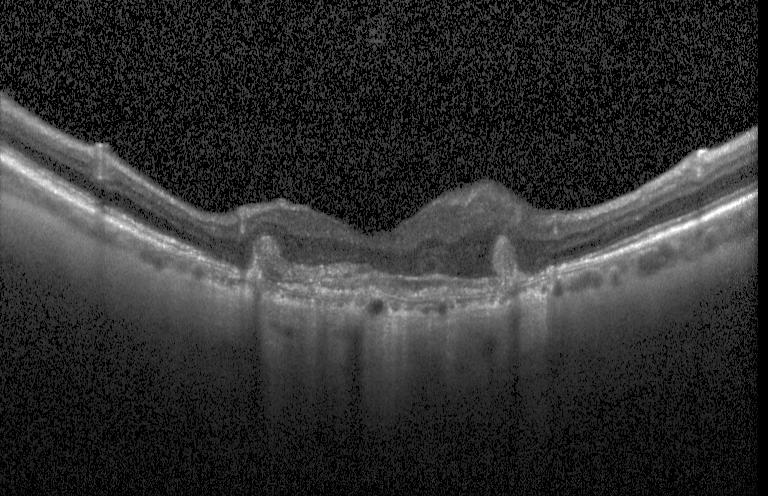
SD-OCT; optical coherence tomography B-scan; horizontal scan through the fovea. CNV.